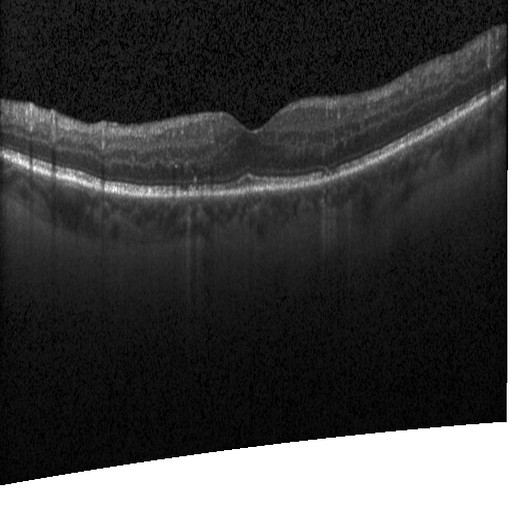 Optical coherence tomography scan; fovea-centered; spectral-domain optical coherence tomography; Heidelberg Spectralis — The scan shows DME.